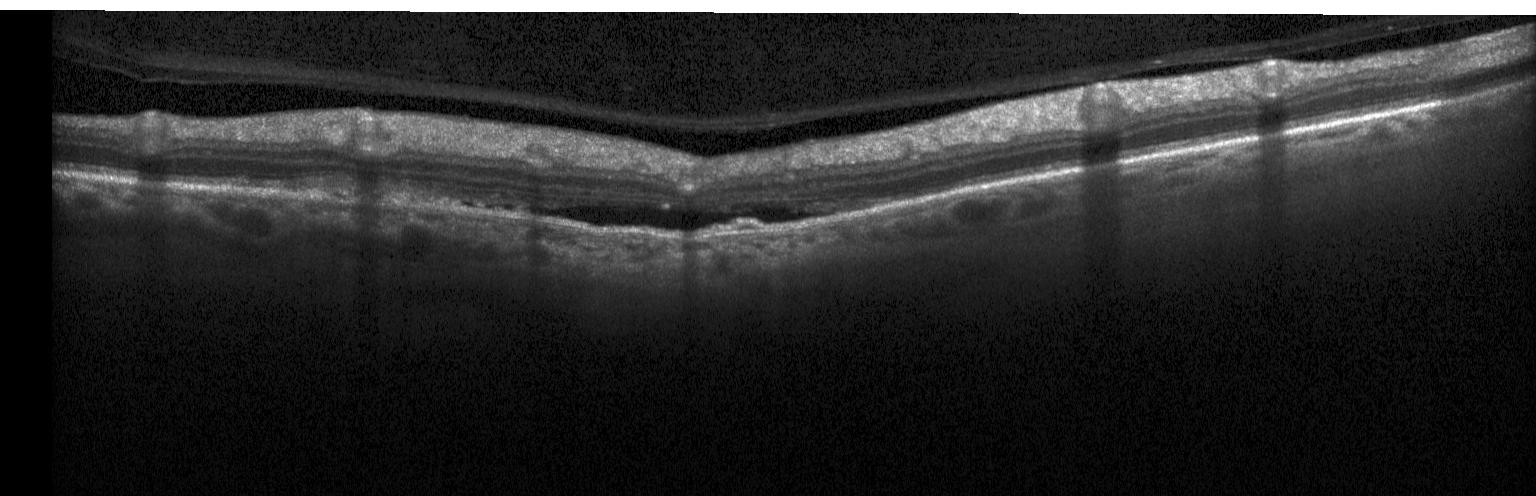

The scan shows choroidal neovascularization (CNV).